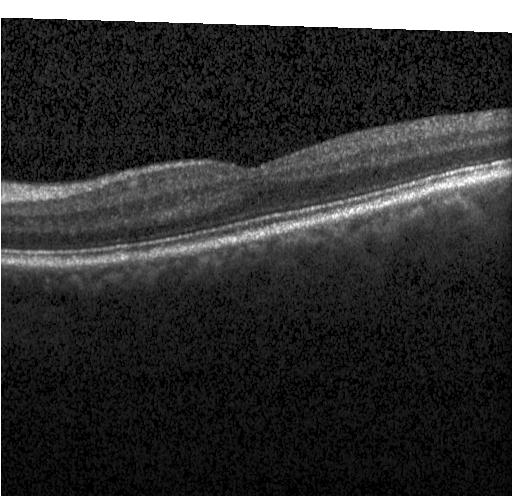

Optical coherence tomography scan — Assessment: neither choroidal neovascularization, diabetic macular edema, nor drusen.